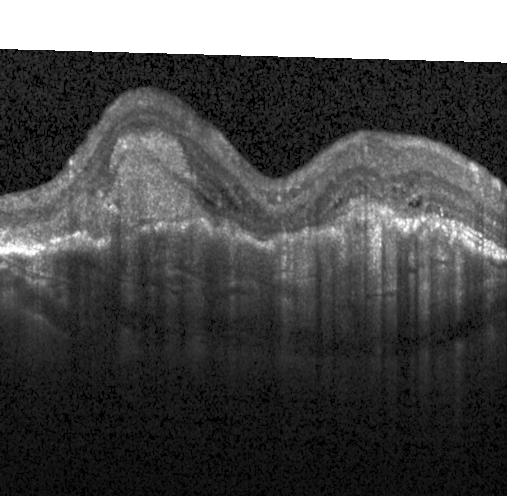 Spectral-domain optical coherence tomography; OCT B-scan; centered on the fovea; Heidelberg Spectralis. A choroidal neovascular membrane.